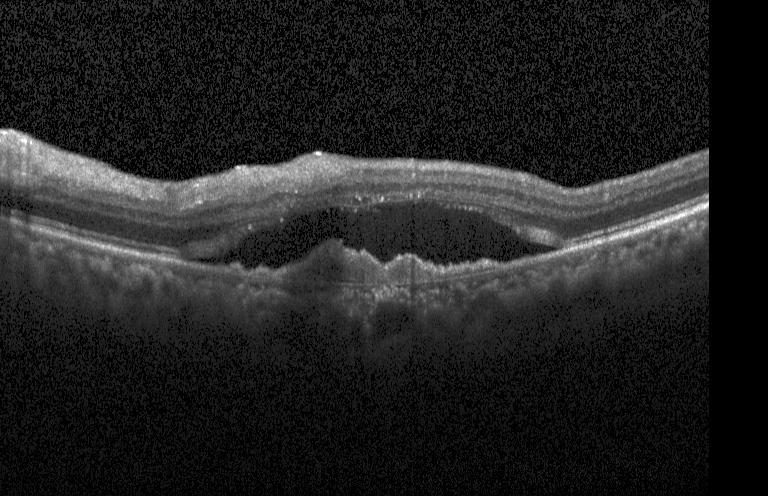
Centered on the fovea, instrument: Heidelberg Spectralis, optical coherence tomography B-scan.
A choroidal neovascular membrane.